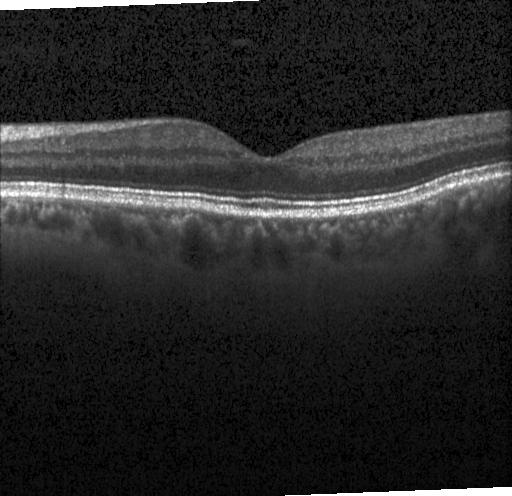
Diagnosis: no choroidal neovascularization, diabetic macular edema, or drusen.